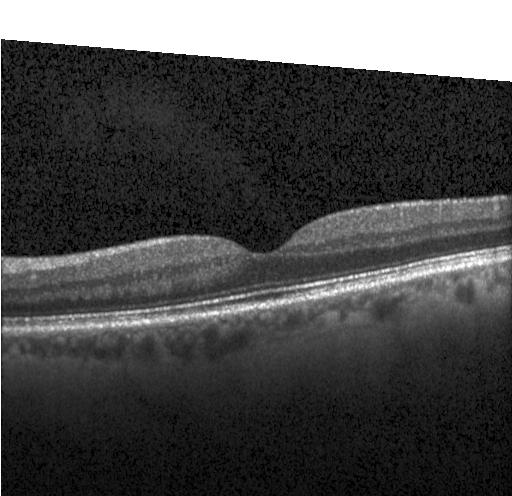

Spectral-domain OCT; OCT line scan.
Diagnosis: no evidence of choroidal neovascularization, diabetic macular edema, or drusen.